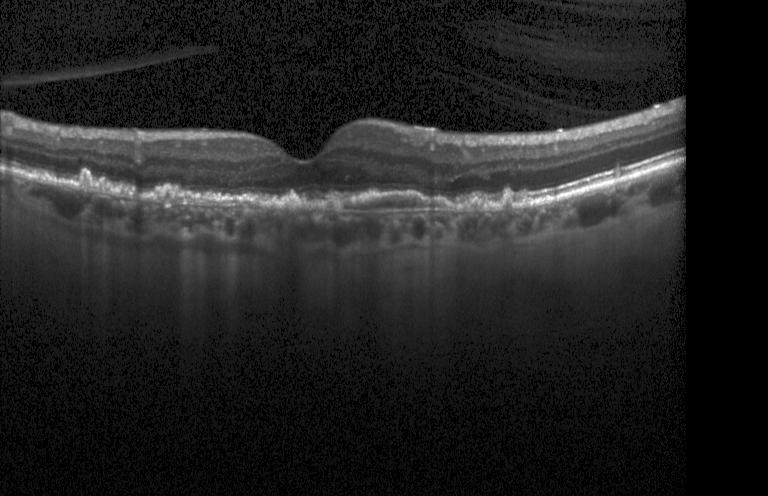
OCT B-scan
Dx: a choroidal neovascular membrane.